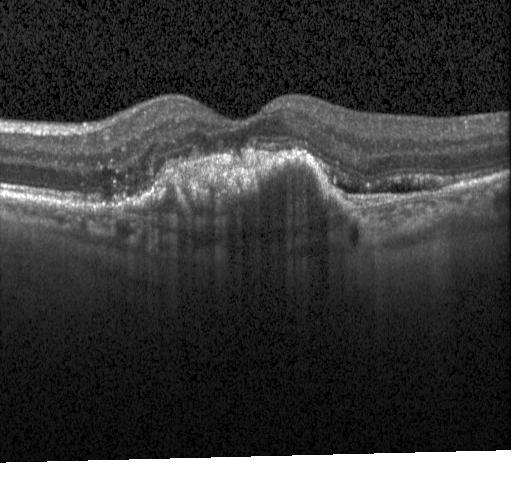
Optical coherence tomography scan.
A choroidal neovascular membrane.